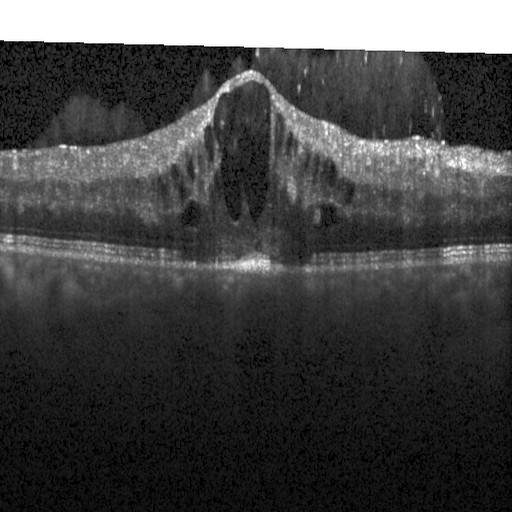

Horizontal scan through the fovea; spectral-domain optical coherence tomography; instrument: Heidelberg Spectralis; optical coherence tomography scan.
Impression: DME.